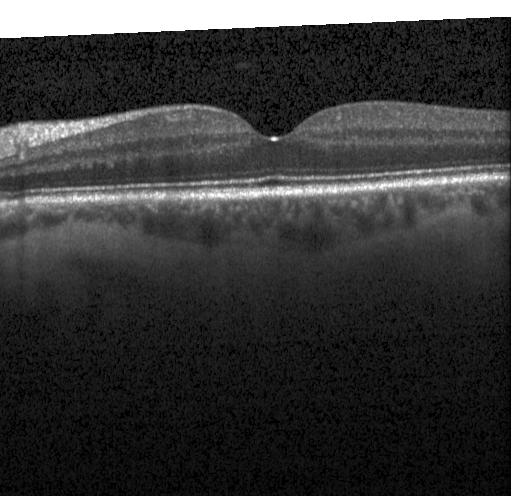
Fovea-centered, optical coherence tomography B-scan, instrument: Heidelberg Spectralis.
Macular OCT: no evidence of CNV, DME, or drusen.